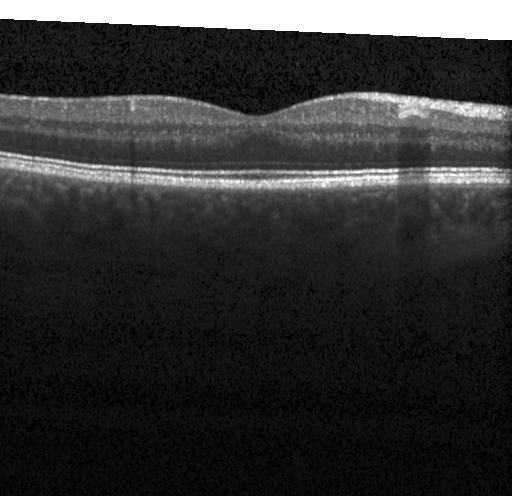 Retinal OCT B-scan; spectral-domain OCT — Macular OCT: no evidence of choroidal neovascularization, diabetic macular edema, or drusen.